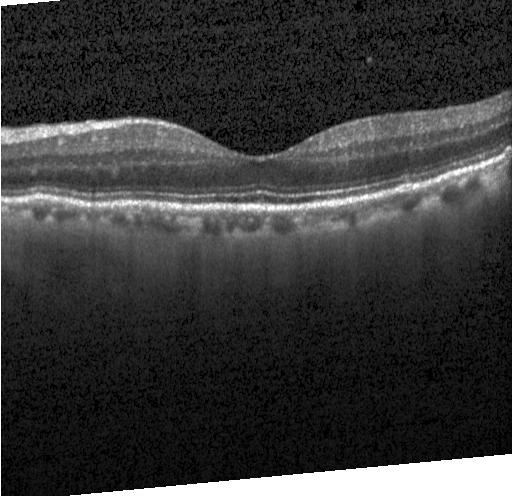

Retinal OCT B-scan — Finding: neither CNV, DME, nor drusen.